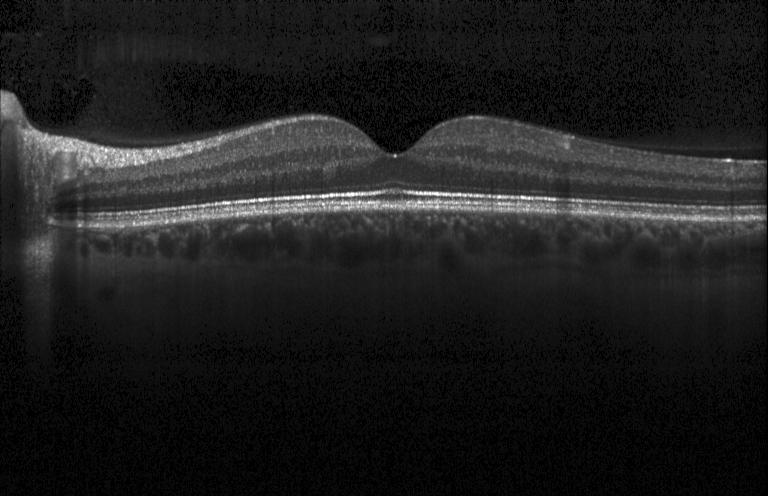 Optical coherence tomography scan. Spectral-domain optical coherence tomography. OCT finding: no CNV, DME, or drusen.